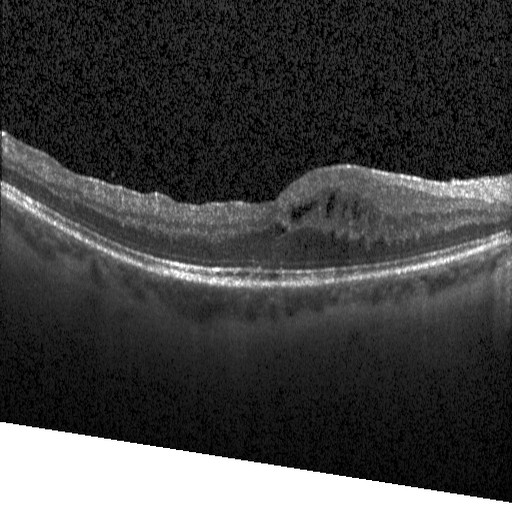

Macular OCT: diabetic macular edema (DME).